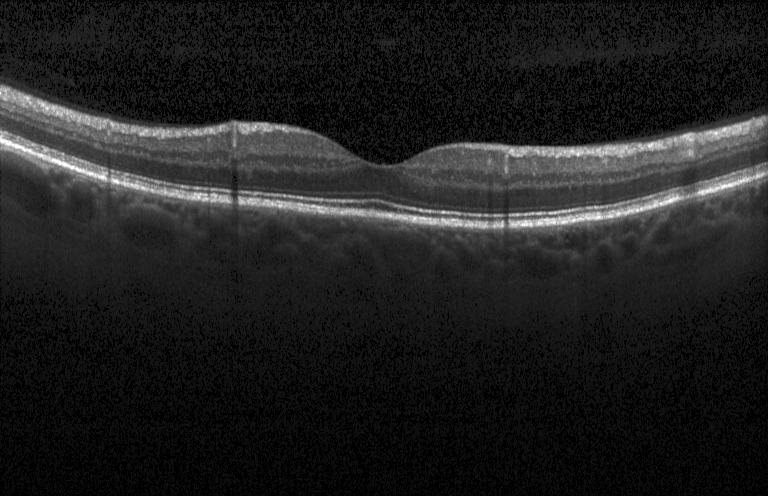

Diagnosis: neither CNV, DME, nor drusen.